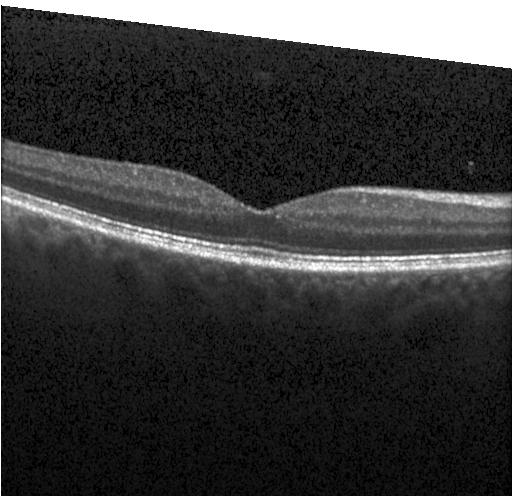 Horizontal scan through the fovea · retinal OCT B-scan · SD-OCT.
Diagnosis: no CNV, DME, or drusen.